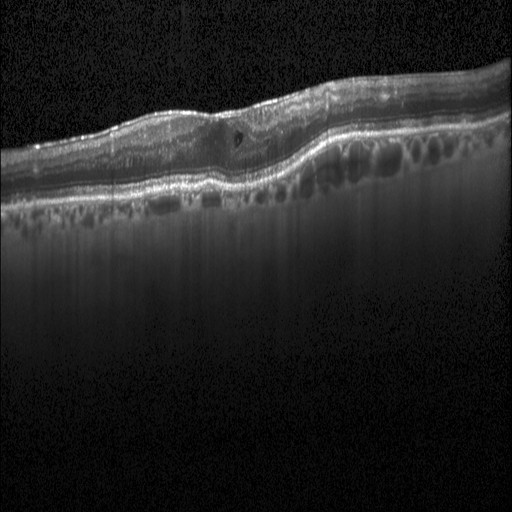

Acquired on a Heidelberg Spectralis; OCT line scan — Finding: diabetic macular edema (DME).